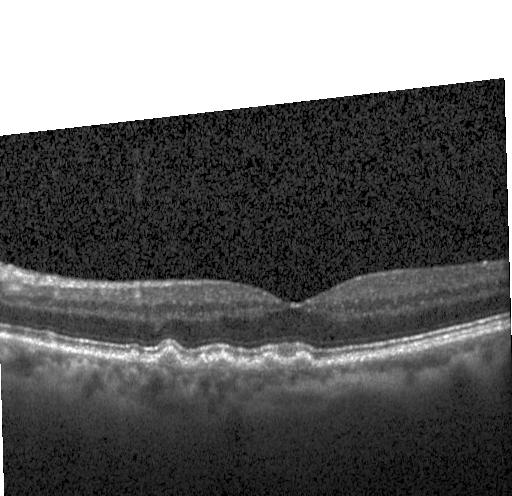

Optical coherence tomography B-scan; spectral-domain OCT; acquired on a Heidelberg Spectralis
This B-scan demonstrates multiple drusen.